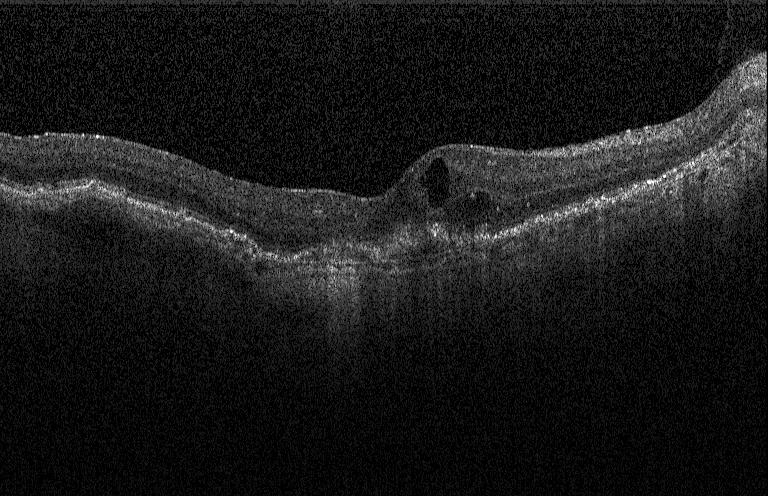 SD-OCT; OCT line scan — Assessment: CNV.